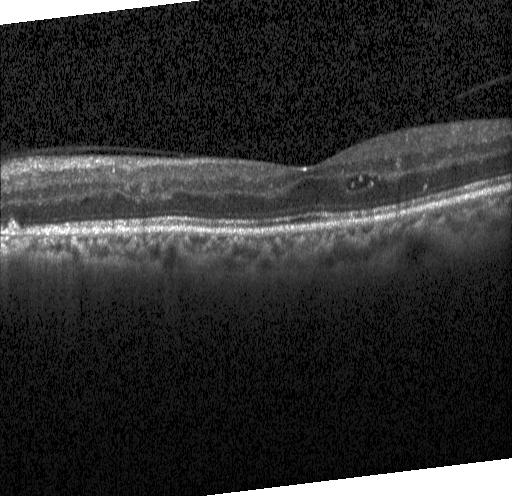

Retinal OCT cross-section; fovea-centered.
Diagnosis: DME.